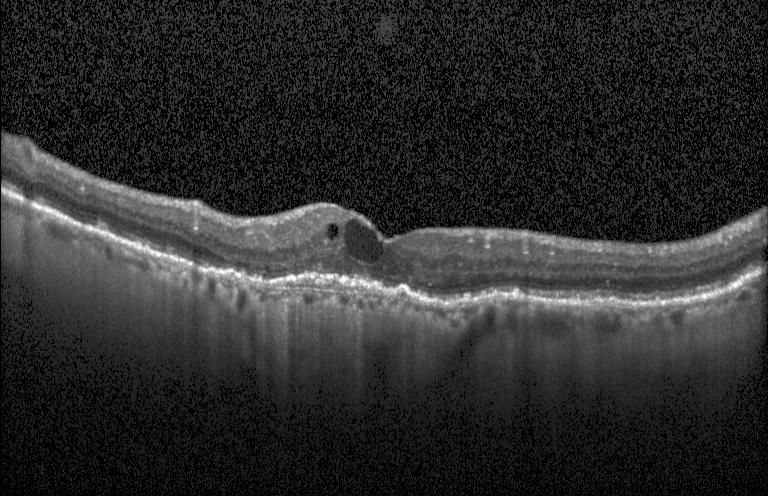

OCT scan showing a choroidal neovascular membrane.